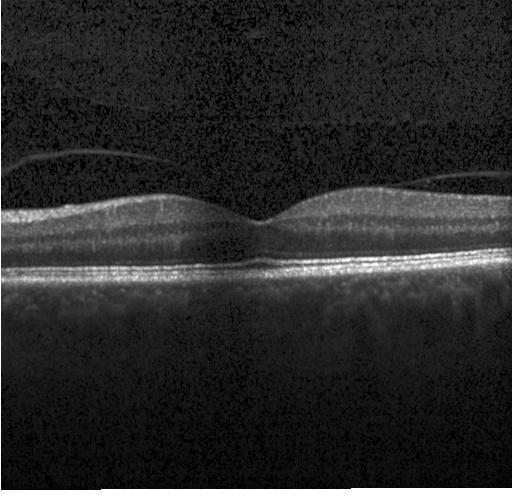

OCT line scan
Impression: no evidence of choroidal neovascularization, diabetic macular edema, or drusen.